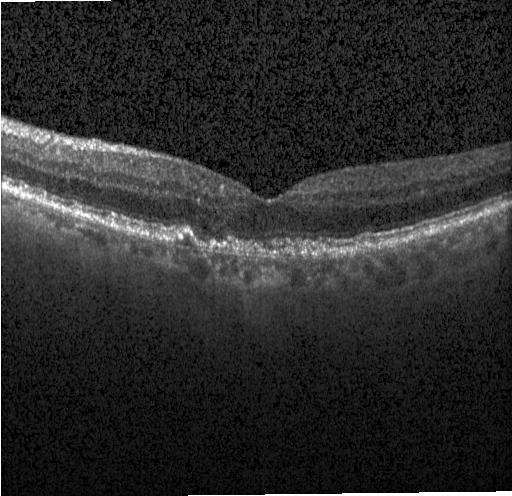

Diagnosis: sub-RPE drusenoid deposits.